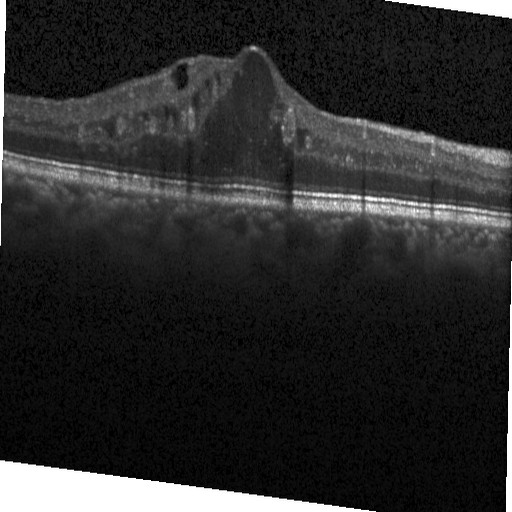

SD-OCT, OCT B-scan, fovea-centered, Heidelberg Spectralis
Diagnosis: diabetic macular edema.